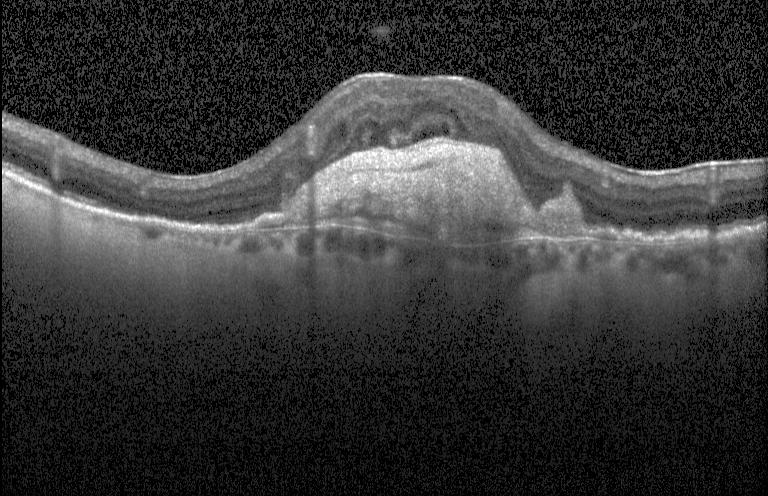
Heidelberg Spectralis; fovea-centered; spectral-domain OCT; retinal OCT cross-section. This B-scan demonstrates a choroidal neovascular membrane.